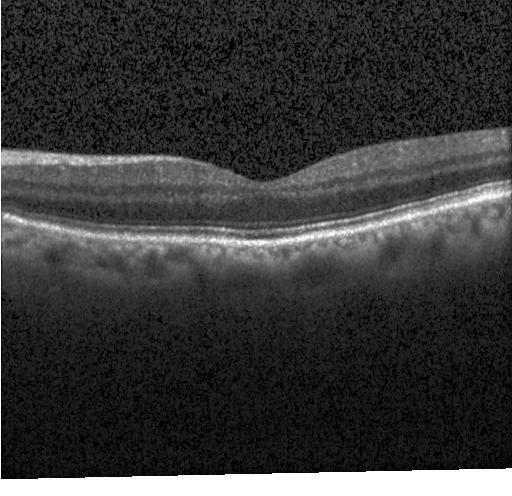
Retinal OCT B-scan.
Assessment: no CNV, no DME, and no drusen.